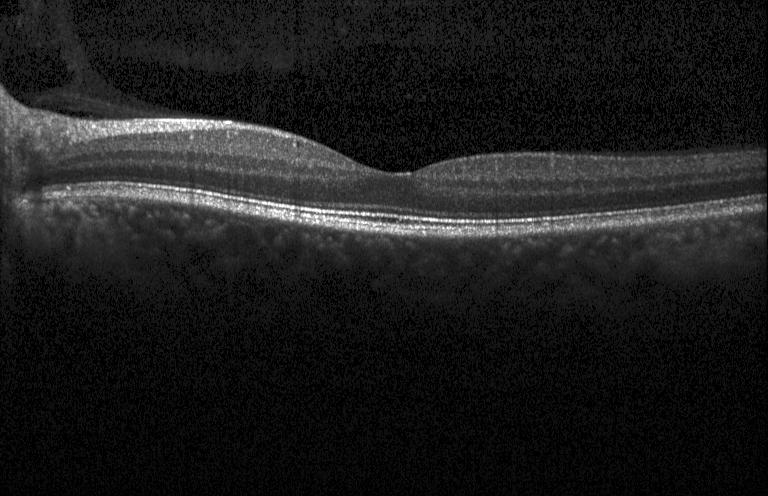 Heidelberg Spectralis. Optical coherence tomography scan — No choroidal neovascularization, diabetic macular edema, or drusen.